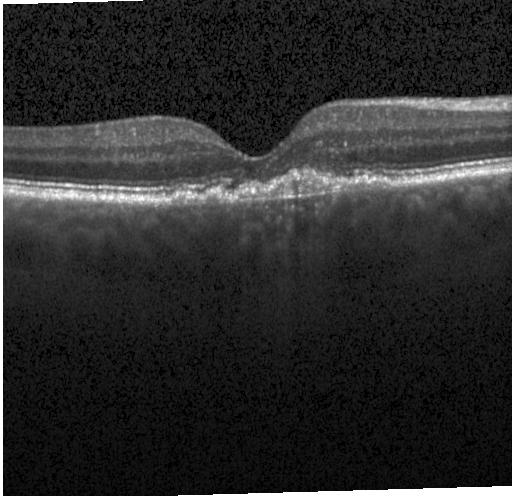
Heidelberg Spectralis. Optical coherence tomography B-scan — Dx: a choroidal neovascular membrane.